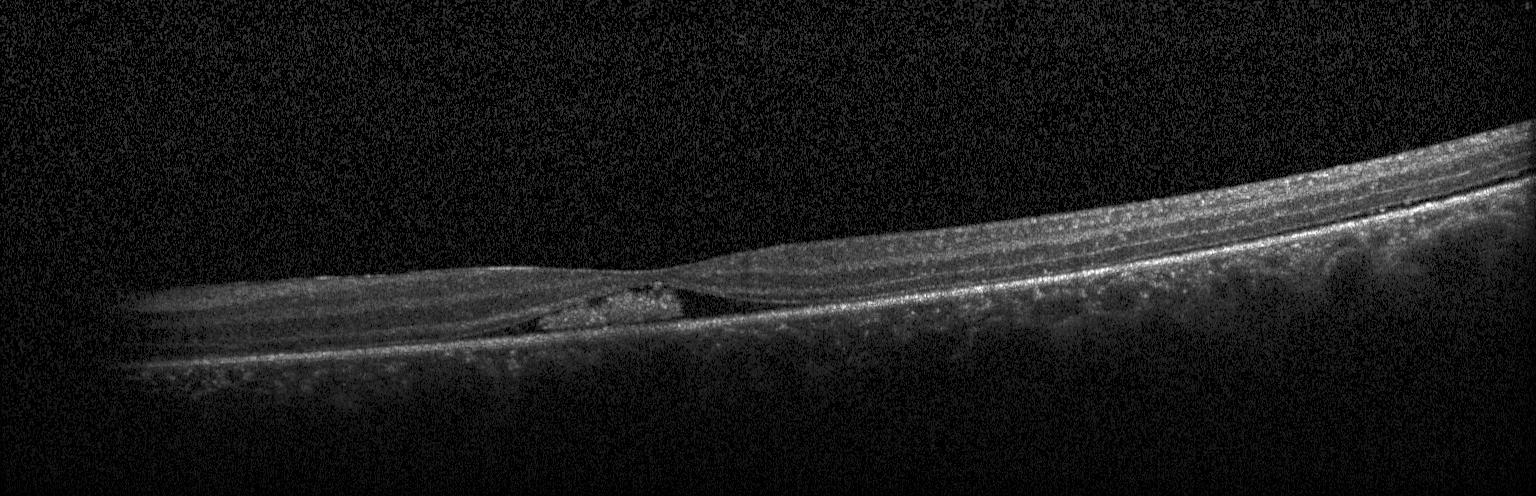
Retinal OCT B-scan. Centered on the fovea — The scan shows a choroidal neovascular membrane.